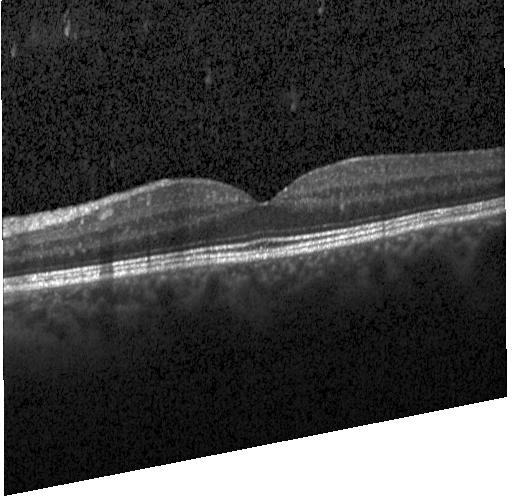

Optical coherence tomography B-scan — Macular OCT: no evidence of choroidal neovascularization, diabetic macular edema, or drusen.